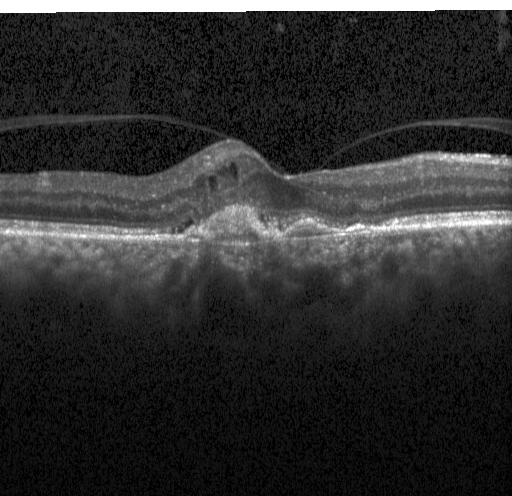 Heidelberg Spectralis · retinal OCT cross-section · spectral-domain OCT.
Diagnosis: choroidal neovascularization.